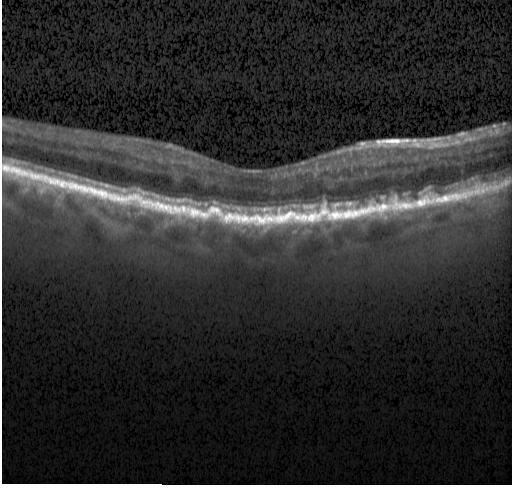 Heidelberg Spectralis OCT system · SD-OCT · through the macula · retinal OCT B-scan — Impression: sub-RPE drusenoid deposits.